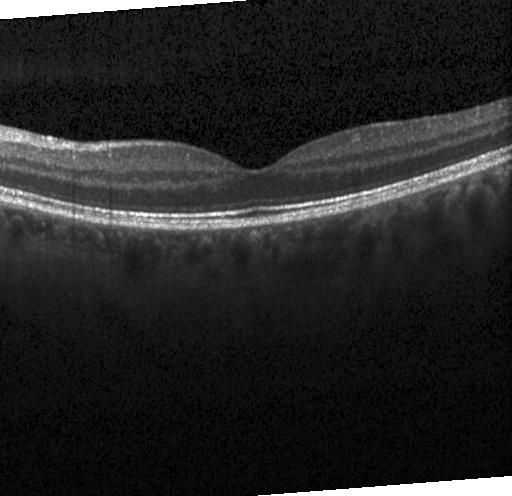
Macular scan · retinal OCT B-scan. Macular OCT: no CNV, no DME, and no drusen.